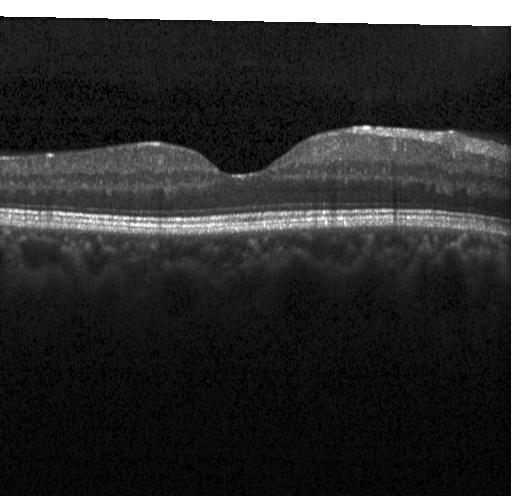
Spectral-domain optical coherence tomography, Heidelberg Spectralis OCT system, optical coherence tomography scan.
No choroidal neovascularization, no diabetic macular edema, and no drusen.